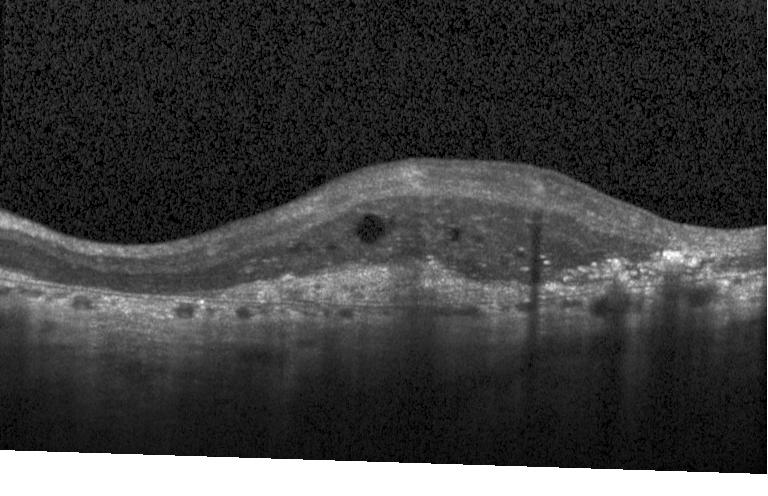
Impression: CNV.